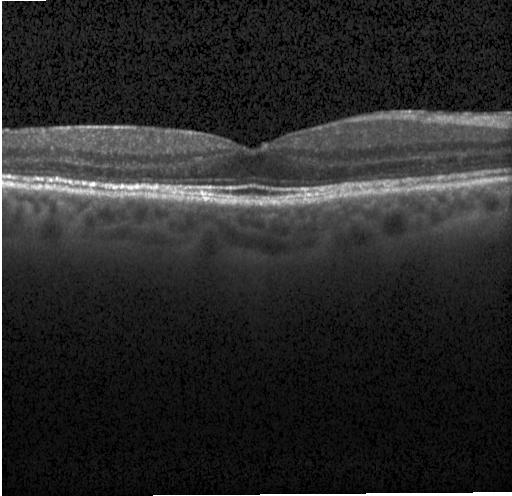

Macular scan; SD-OCT; Heidelberg Spectralis; retinal OCT cross-section.
No evidence of choroidal neovascularization, diabetic macular edema, or drusen.